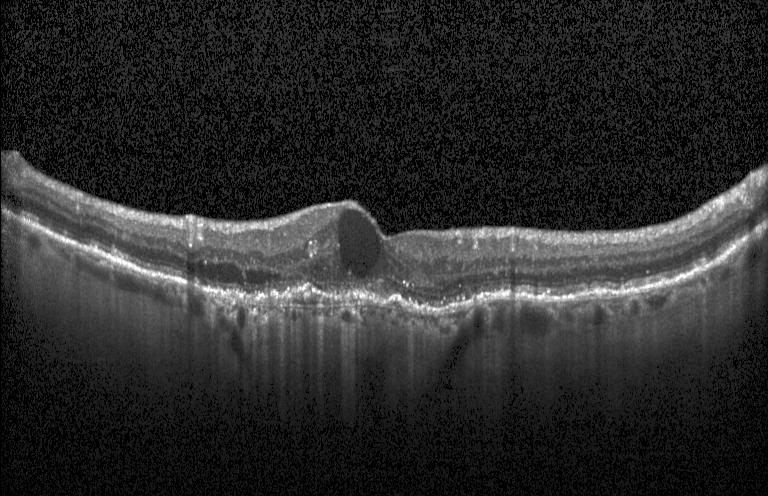

OCT B-scan showing choroidal neovascularization (CNV).